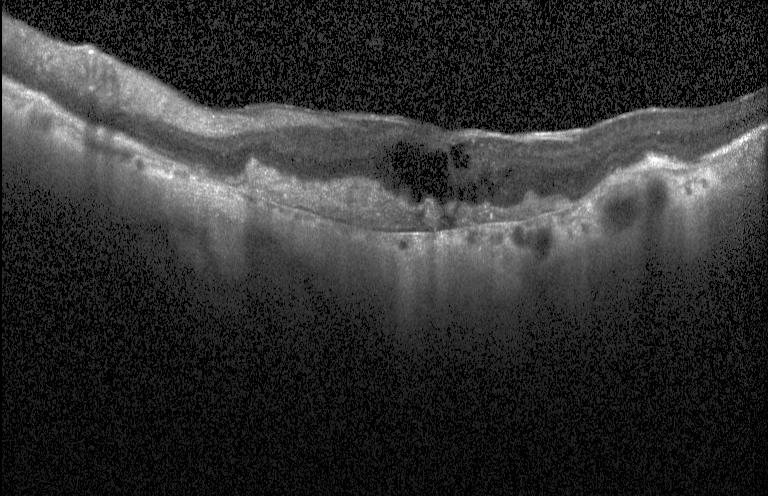 Retinal OCT cross-section — Assessment: a choroidal neovascular membrane.